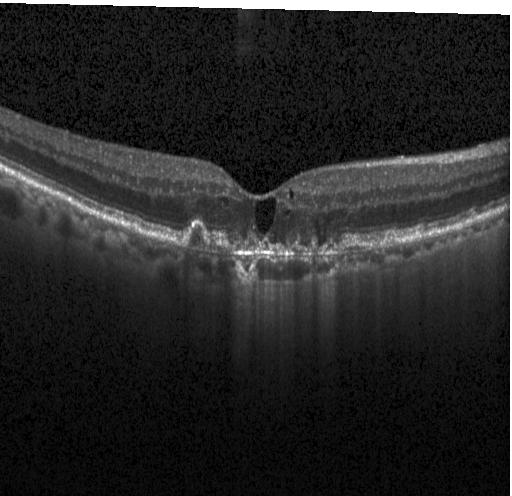
Horizontal scan through the fovea, acquired on a Heidelberg Spectralis, SD-OCT, retinal OCT B-scan. Choroidal neovascularization.